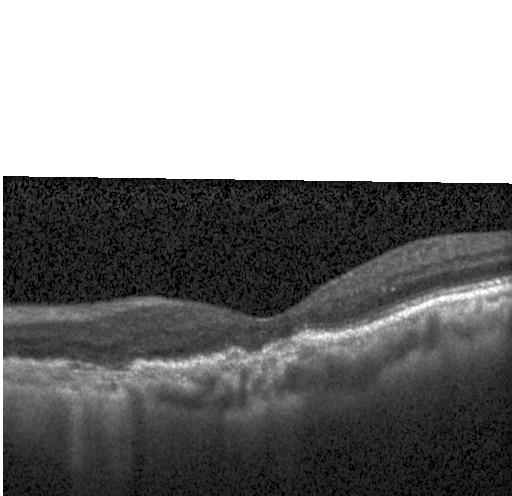 Optical coherence tomography B-scan
This B-scan demonstrates a choroidal neovascular membrane.